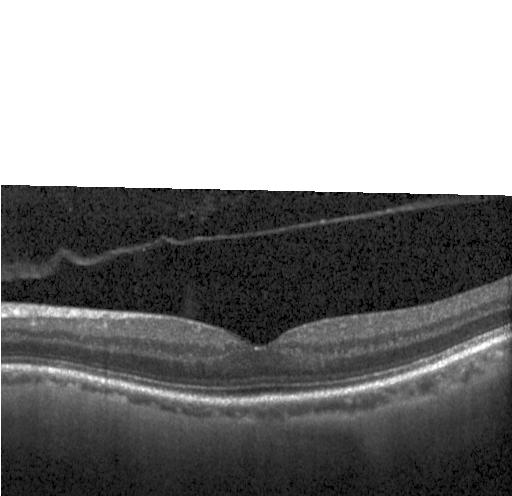 Horizontal scan through the fovea; spectral-domain optical coherence tomography; OCT line scan; Heidelberg Spectralis OCT system — This B-scan demonstrates no evidence of CNV, DME, or drusen.